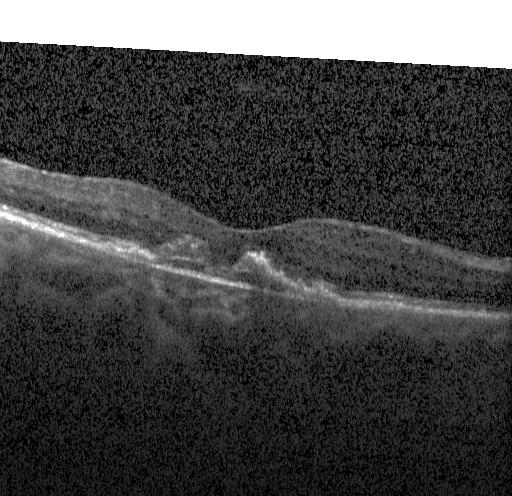
Impression: choroidal neovascularization (CNV).